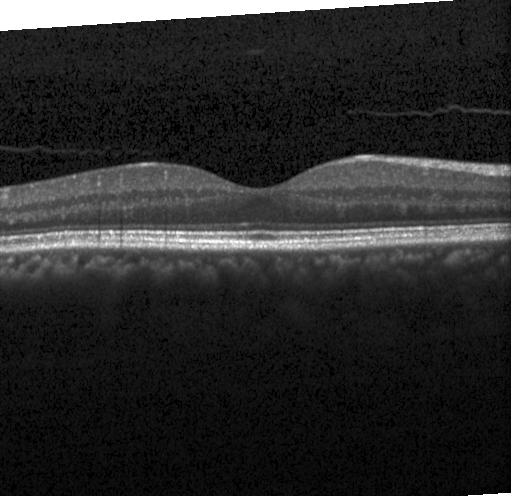
Dx: no choroidal neovascularization, diabetic macular edema, or drusen.